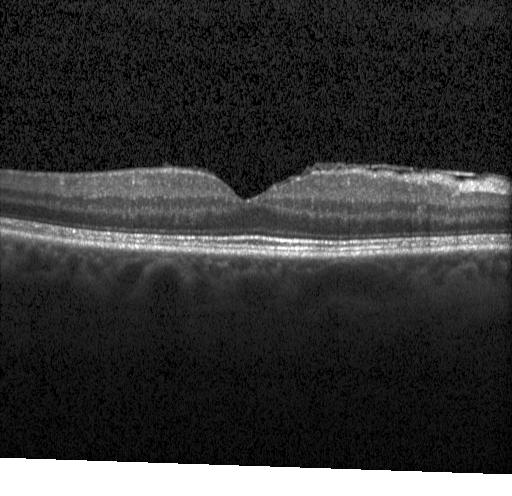

Optical coherence tomography B-scan · instrument: Heidelberg Spectralis · centered on the fovea.
No CNV, no DME, and no drusen.